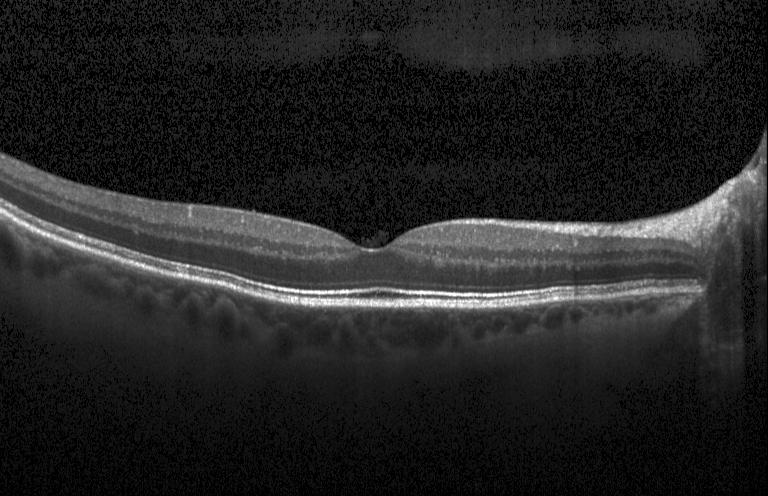
OCT B-scan showing no evidence of choroidal neovascularization, diabetic macular edema, or drusen.